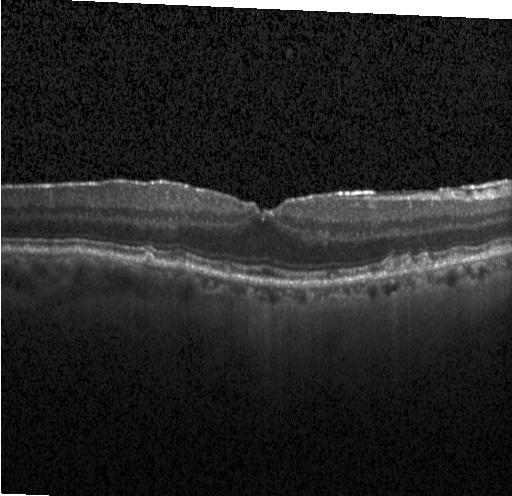 Optical coherence tomography B-scan. This B-scan demonstrates drusen.